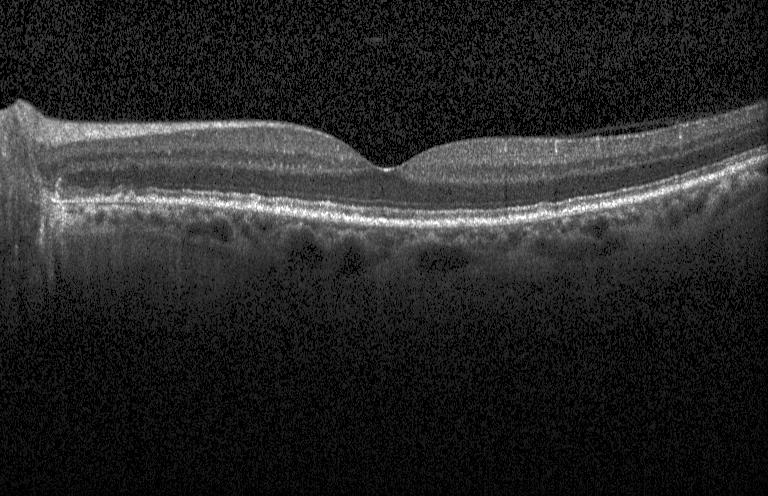
Instrument: Heidelberg Spectralis. Optical coherence tomography scan — Impression: no evidence of choroidal neovascularization, diabetic macular edema, or drusen.